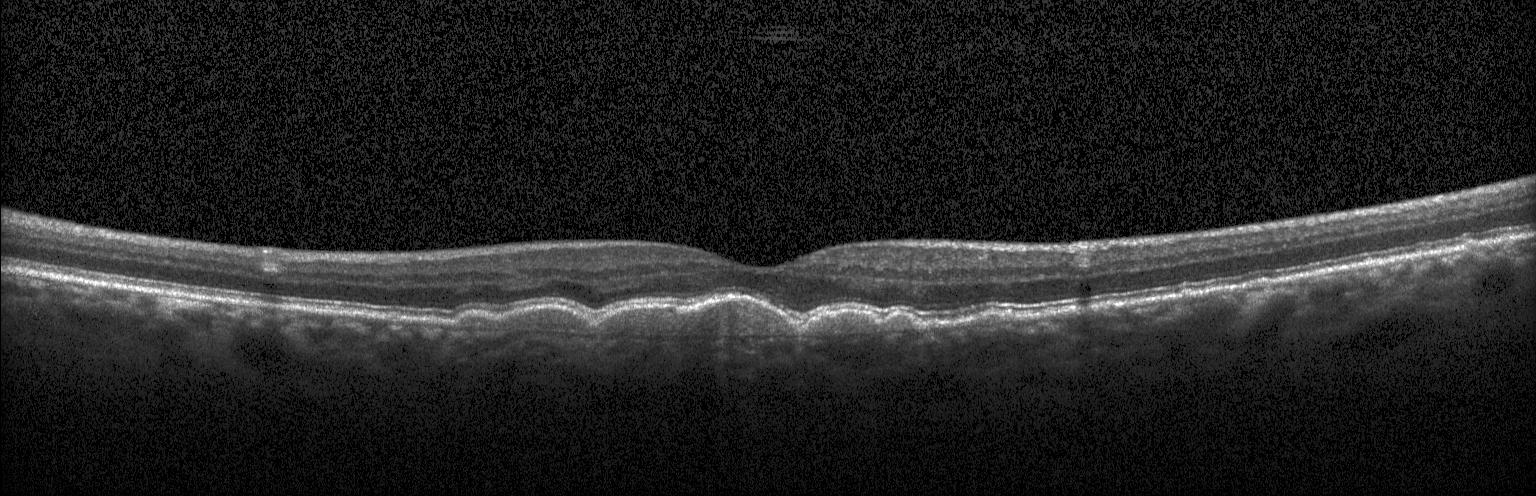

OCT scan showing a choroidal neovascular membrane.